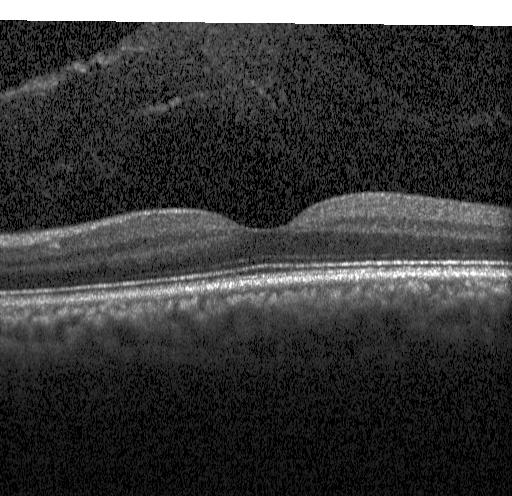 Finding: no evidence of CNV, DME, or drusen.